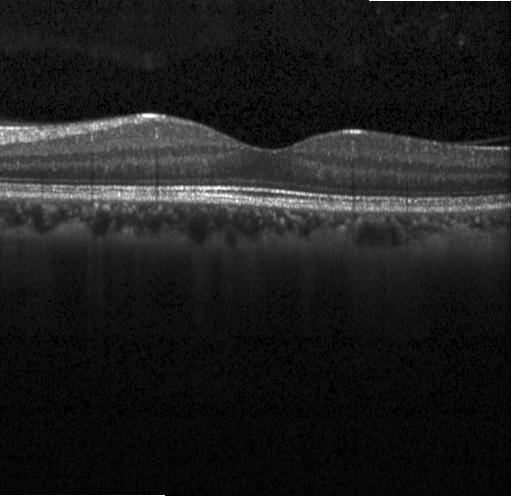 Heidelberg Spectralis OCT system. Through the macula. Spectral-domain optical coherence tomography. Optical coherence tomography scan
Dx: no evidence of CNV, DME, or drusen.